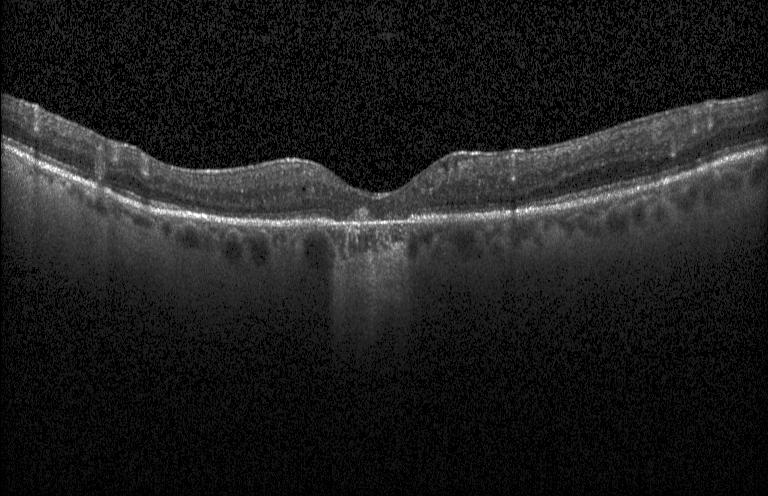
Impression: a choroidal neovascular membrane.